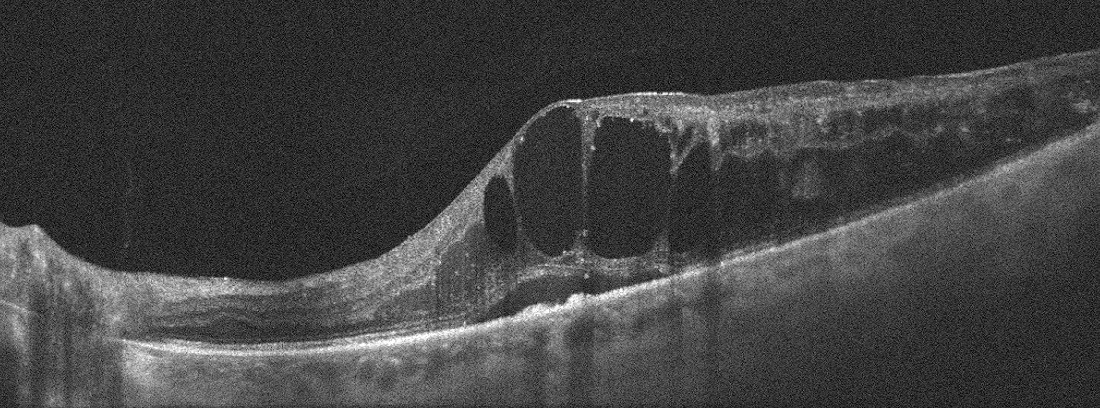

OCT line scan — Impression: RVO.